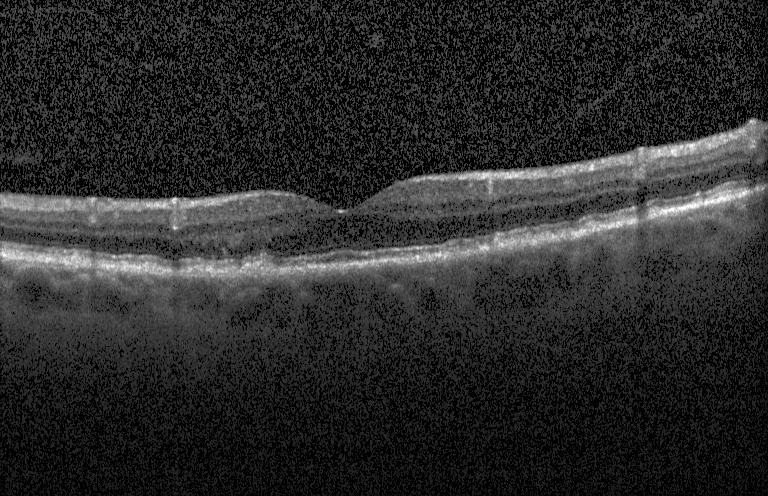

Diagnosis: drusen.